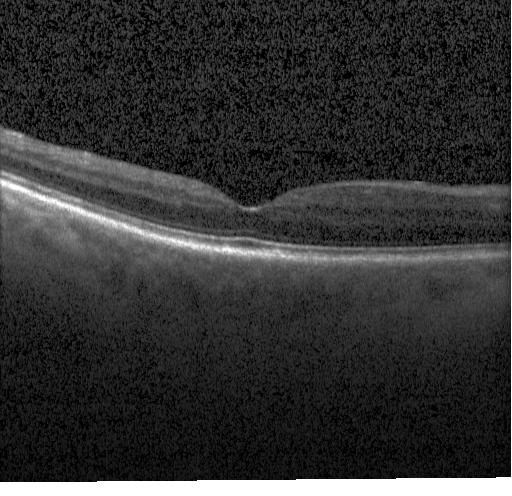
This B-scan demonstrates no choroidal neovascularization, no diabetic macular edema, and no drusen.